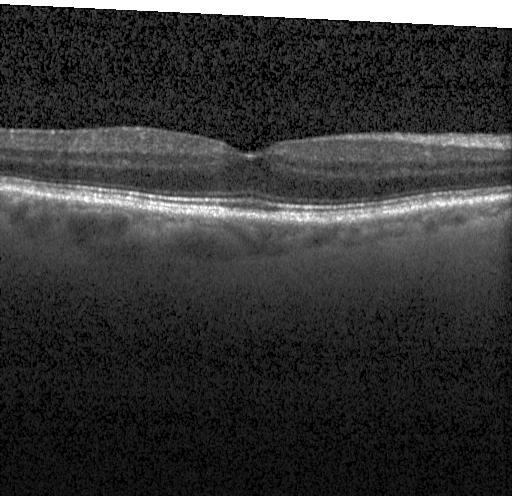
Heidelberg Spectralis. Retinal OCT B-scan
OCT finding: no choroidal neovascularization, diabetic macular edema, or drusen.